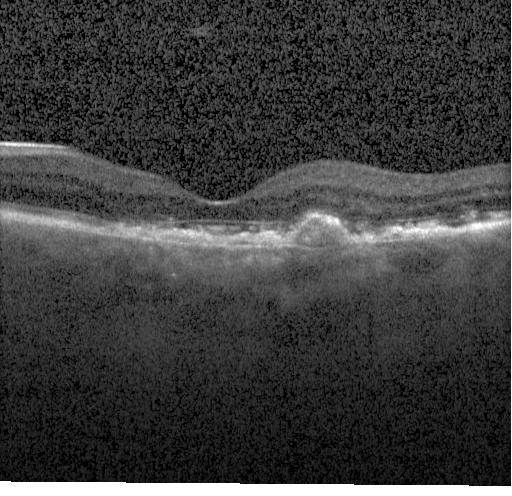
Macular OCT: a choroidal neovascular membrane.